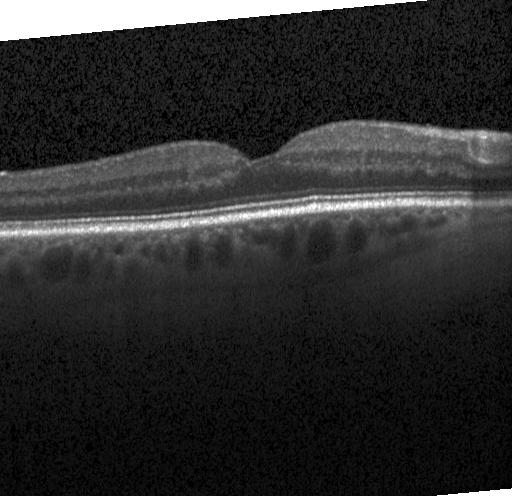
Macular OCT demonstrating neither CNV, DME, nor drusen.